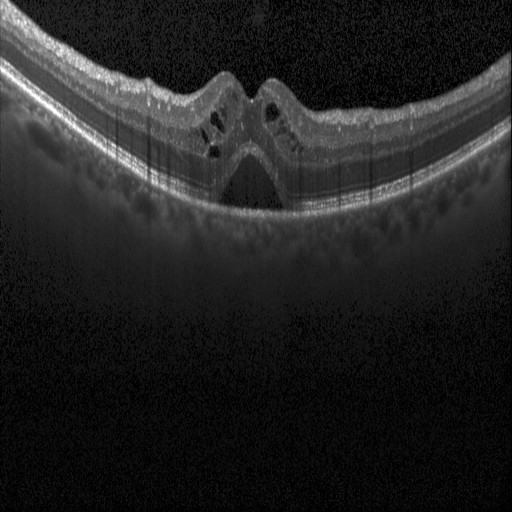 Heidelberg Spectralis OCT system. Optical coherence tomography B-scan. Fovea-centered. Spectral-domain optical coherence tomography. Finding: diabetic macular edema.